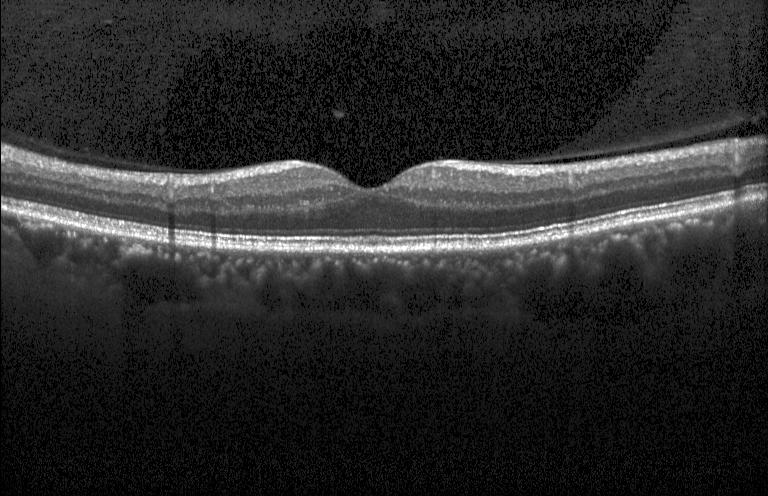
OCT B-scan showing no choroidal neovascularization, diabetic macular edema, or drusen.